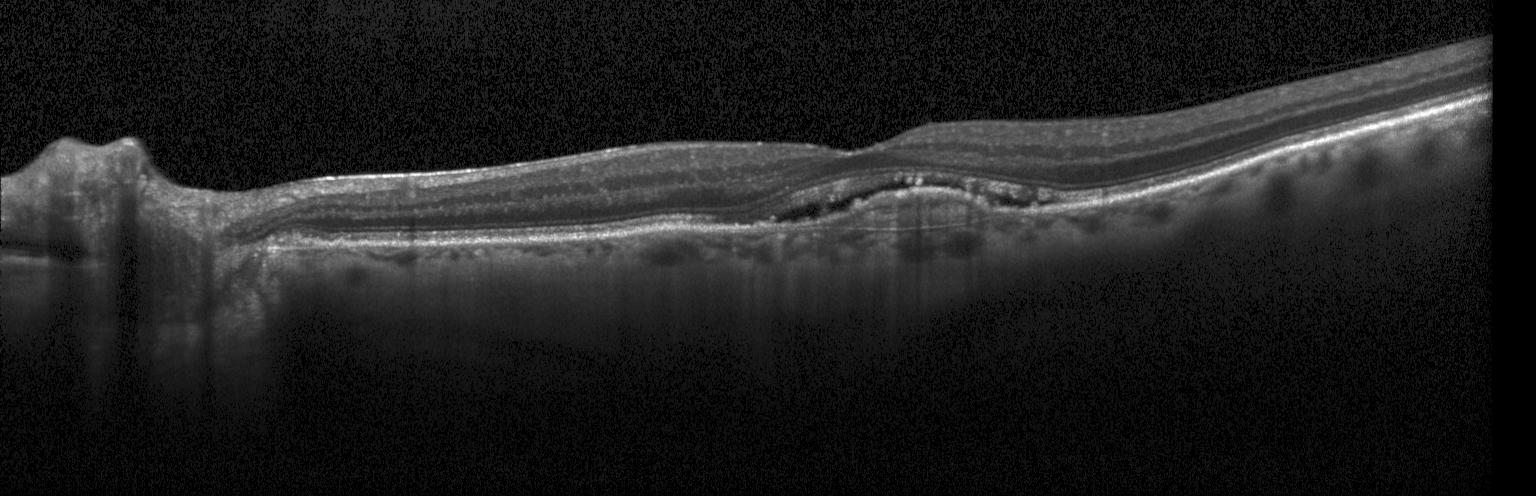
SD-OCT. Retinal OCT B-scan. Centered on the fovea — Macular OCT: choroidal neovascularization.